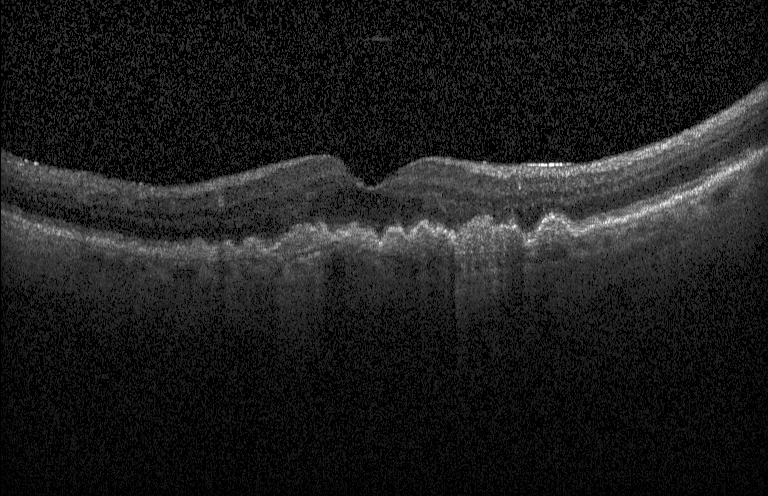 Spectral-domain OCT · optical coherence tomography B-scan · centered on the fovea · Heidelberg Spectralis OCT system
OCT finding: sub-RPE drusenoid deposits.